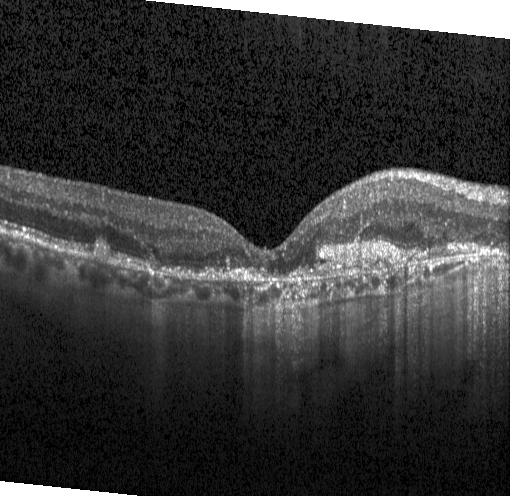 Retinal OCT B-scan, SD-OCT, Heidelberg Spectralis.
Impression: a choroidal neovascular membrane.